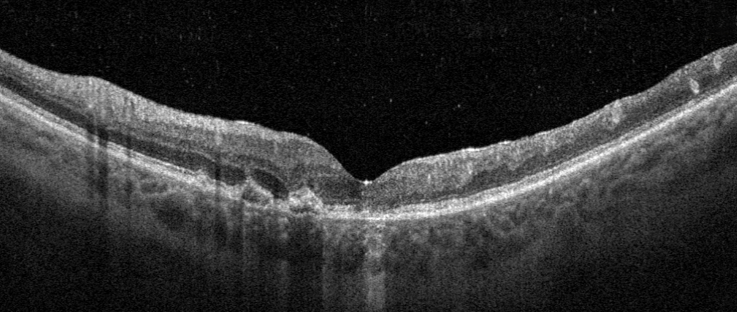
Spectral-domain OCT B-scan: diabetic macular edema.